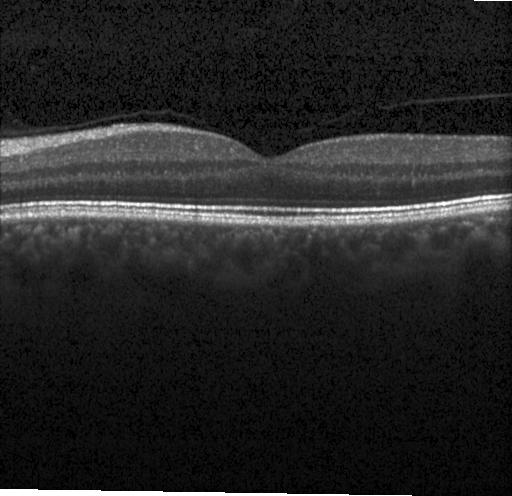

Diagnosis: no choroidal neovascularization, no diabetic macular edema, and no drusen.